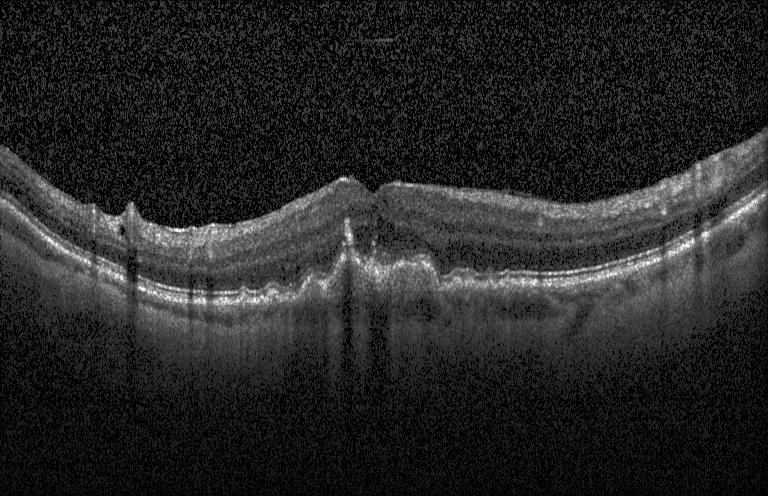 Diagnosis: multiple drusen.